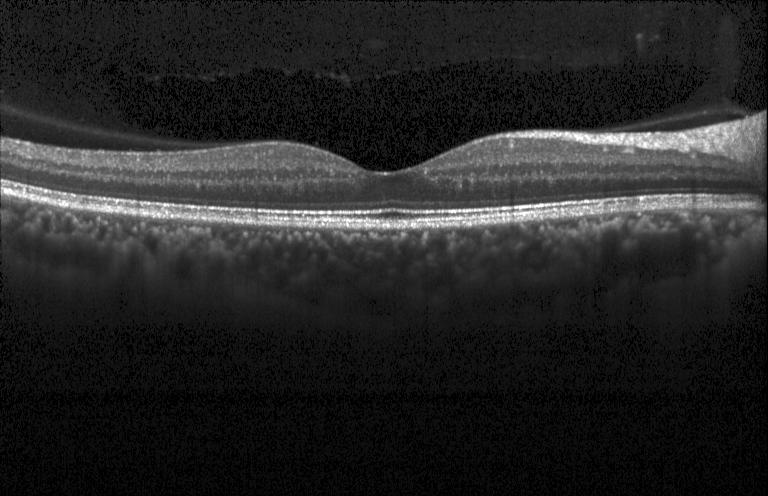
Retinal OCT cross-section — Impression: no CNV, DME, or drusen.